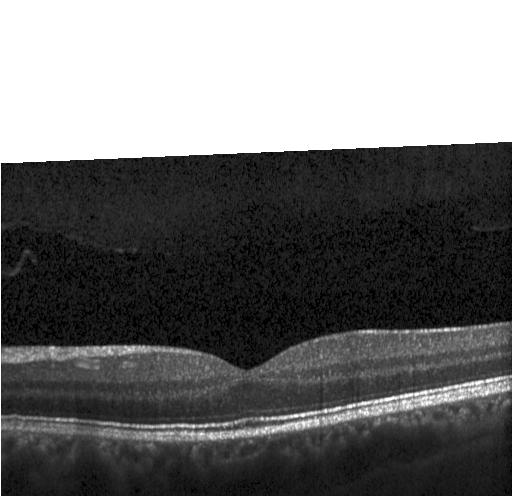 Impression: no choroidal neovascularization, diabetic macular edema, or drusen.